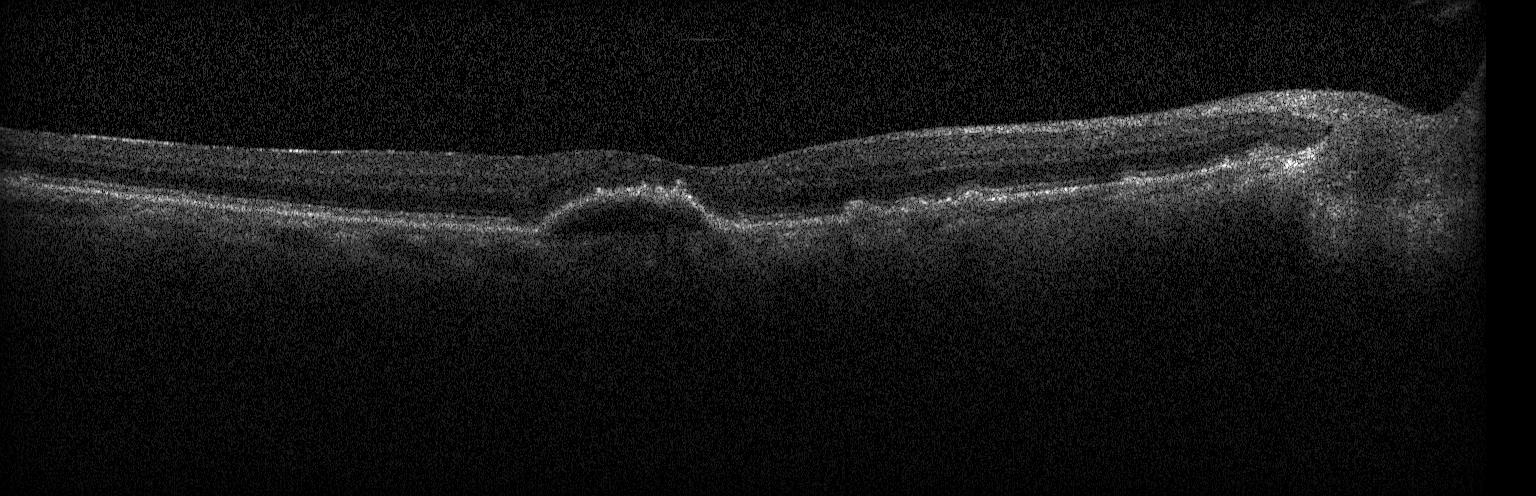
Retinal OCT cross-section showing choroidal neovascularization (CNV).